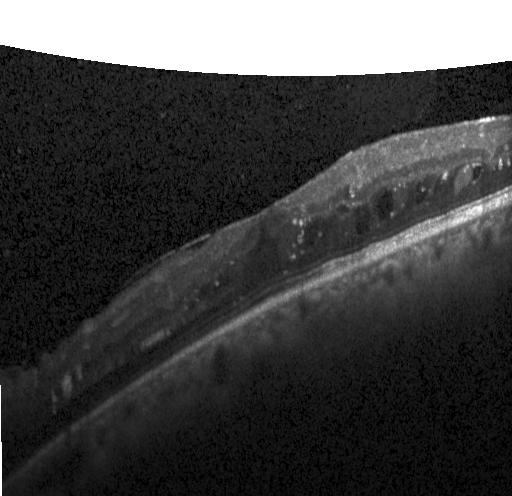 Diagnosis: diabetic macular edema (DME).